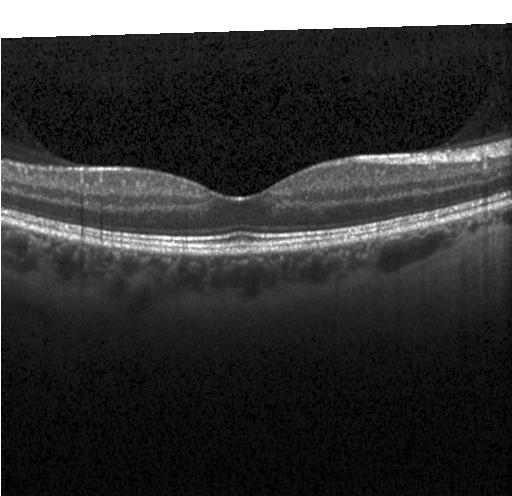
OCT line scan — Finding: no choroidal neovascularization, no diabetic macular edema, and no drusen.